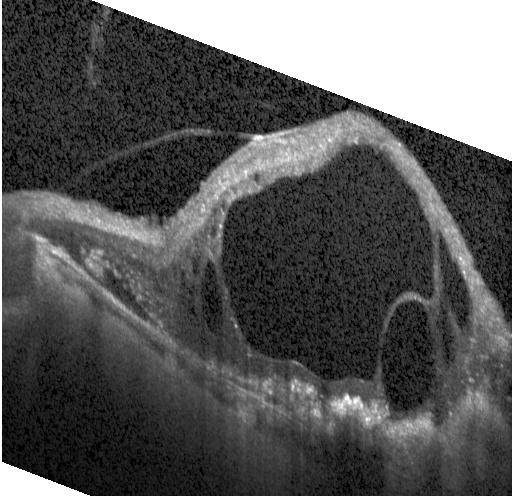
Spectral-domain OCT B-scan: CNV.